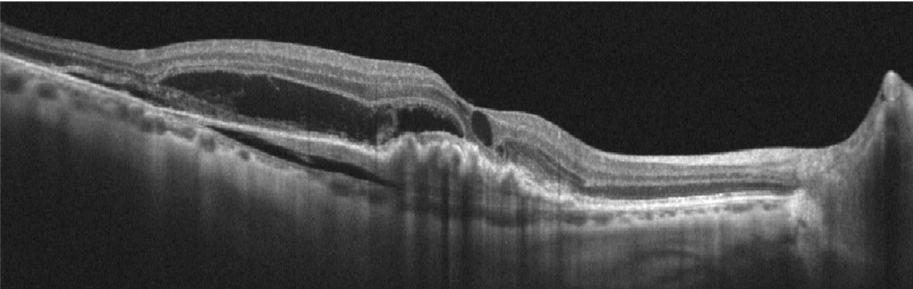
Diagnosis: age-related macular degeneration.